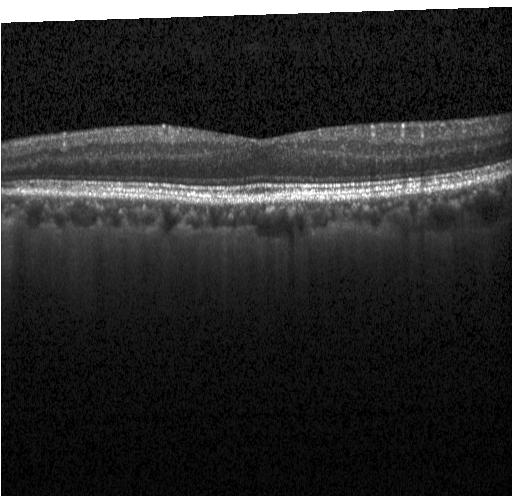 Acquired on a Heidelberg Spectralis, fovea-centered, spectral-domain optical coherence tomography, OCT line scan.
Diagnosis: neither choroidal neovascularization, diabetic macular edema, nor drusen.